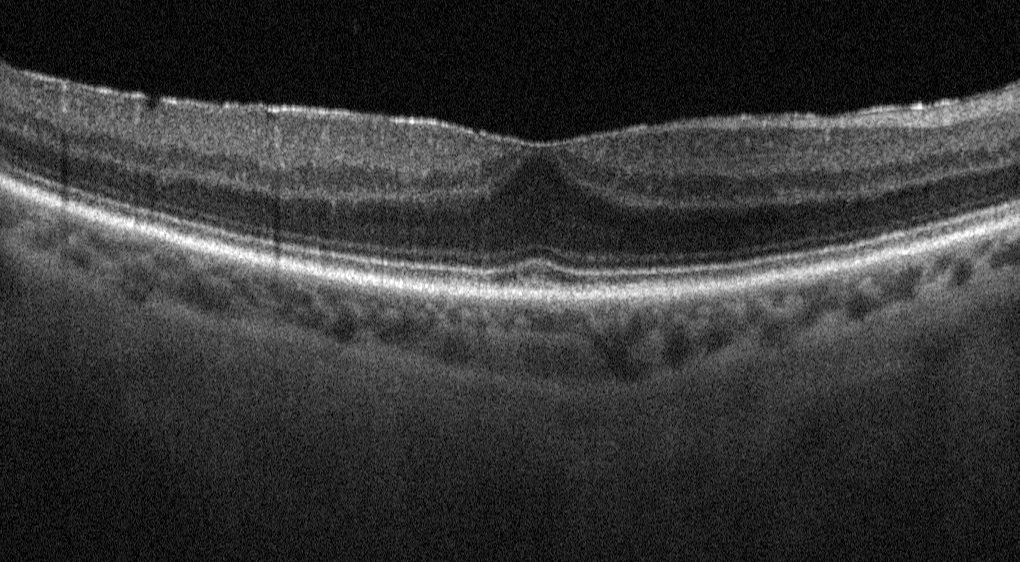

Retinal OCT cross-section — Dx: ERM.